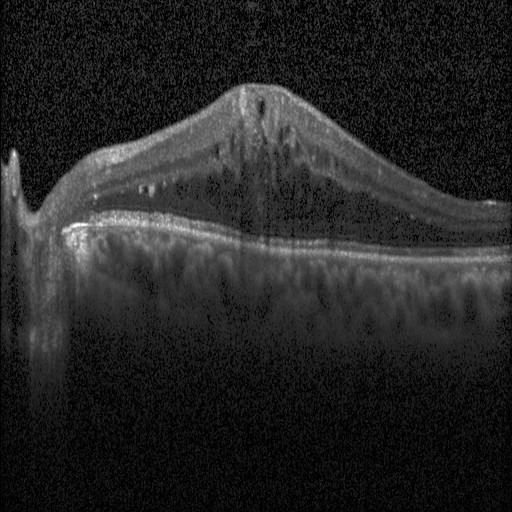 Spectral-domain optical coherence tomography; macular scan; optical coherence tomography B-scan
Finding: diabetic macular edema.